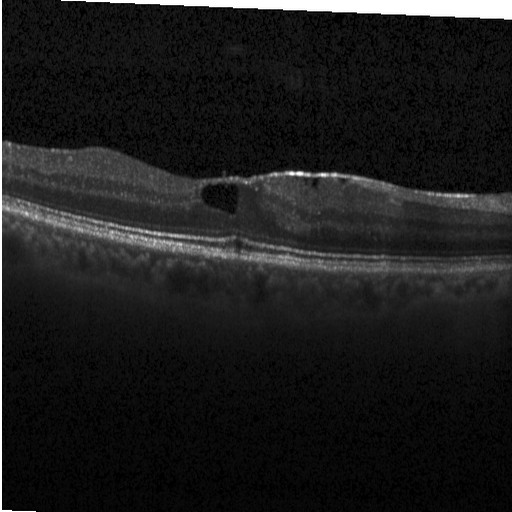 Through the macula, retinal OCT B-scan. Finding: DME.